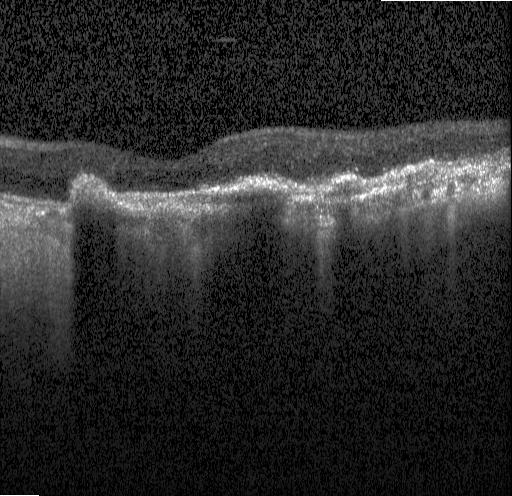 Centered on the fovea; retinal OCT B-scan.
Choroidal neovascularization (CNV).